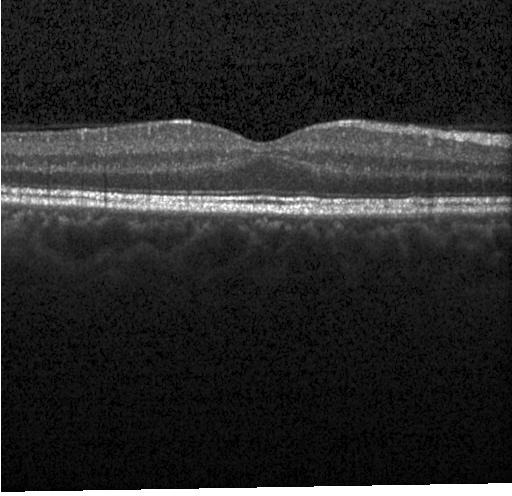 Retinal OCT cross-section showing no choroidal neovascularization, diabetic macular edema, or drusen.